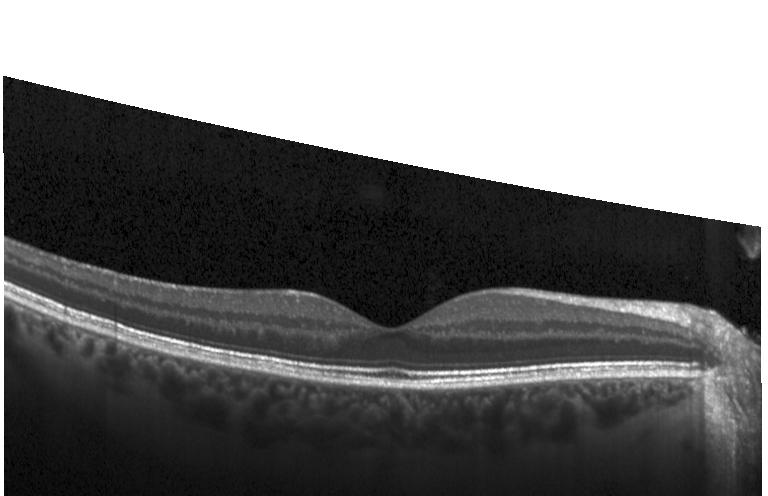 OCT scan showing no choroidal neovascularization, no diabetic macular edema, and no drusen.